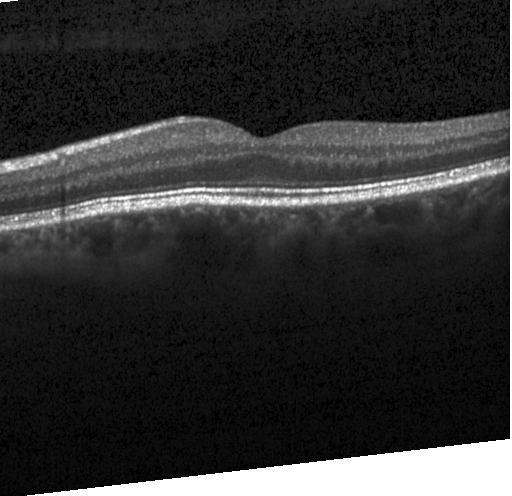

Fovea-centered; SD-OCT; Heidelberg Spectralis; retinal OCT B-scan. Assessment: no evidence of CNV, DME, or drusen.